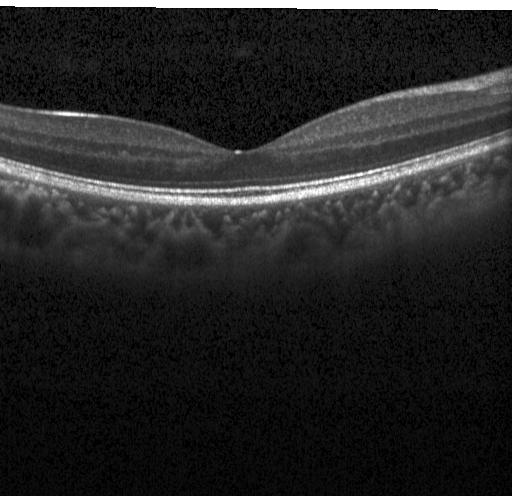
Retinal OCT cross-section · spectral-domain OCT · instrument: Heidelberg Spectralis.
This B-scan demonstrates neither choroidal neovascularization, diabetic macular edema, nor drusen.